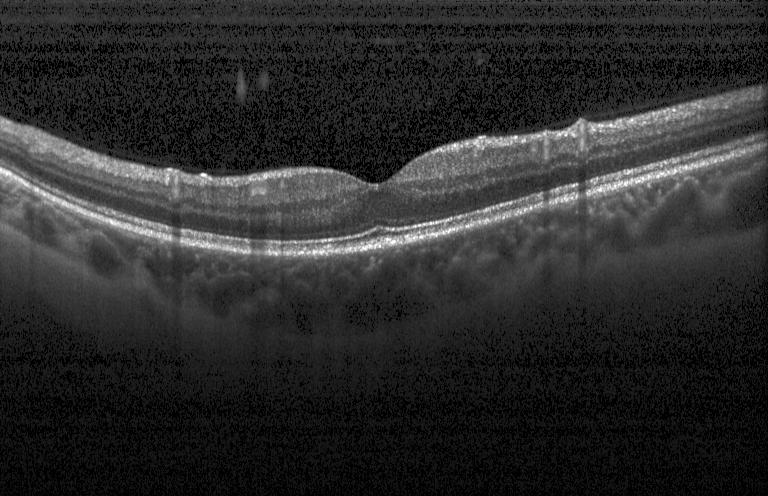
Horizontal scan through the fovea · Heidelberg Spectralis · optical coherence tomography B-scan — Finding: no CNV, no DME, and no drusen.